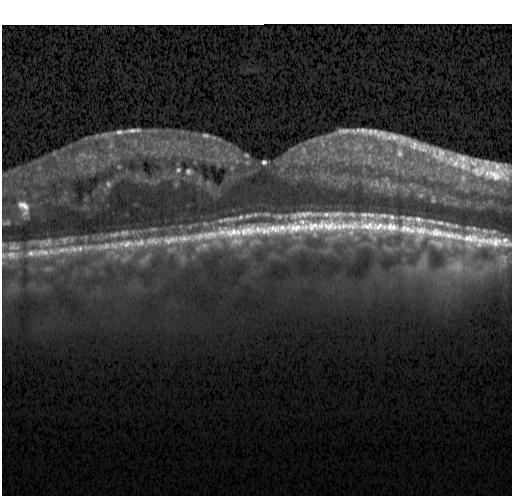
Centered on the fovea; OCT B-scan; spectral-domain optical coherence tomography; acquired on a Heidelberg Spectralis — Macular OCT: DME.